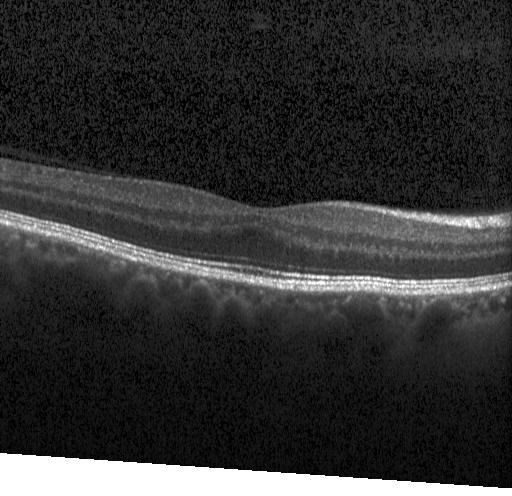 Horizontal scan through the fovea. OCT line scan. Acquired on a Heidelberg Spectralis.
No choroidal neovascularization, diabetic macular edema, or drusen.